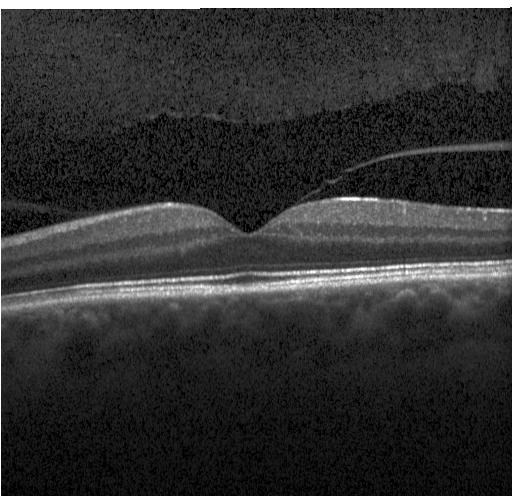

Fovea-centered · OCT line scan.
Dx: no choroidal neovascularization, diabetic macular edema, or drusen.